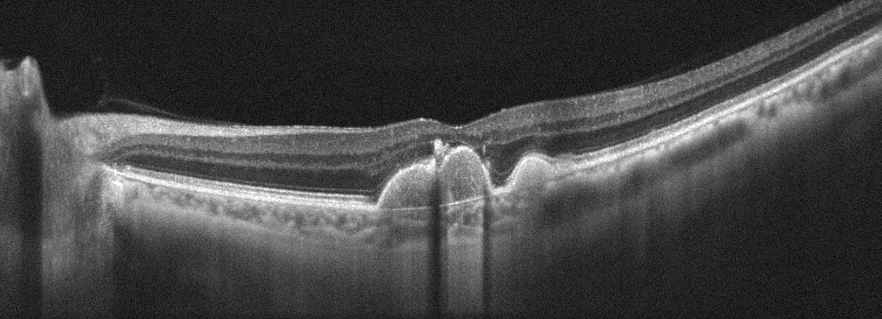

OS, optical coherence tomography scan.
Finding: age-related macular degeneration (AMD).